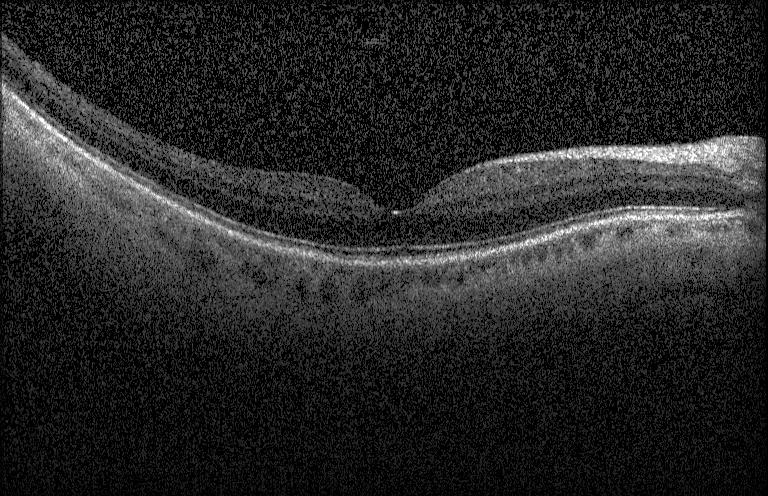

Retinal OCT cross-section · centered on the fovea. Dx: neither choroidal neovascularization, diabetic macular edema, nor drusen.